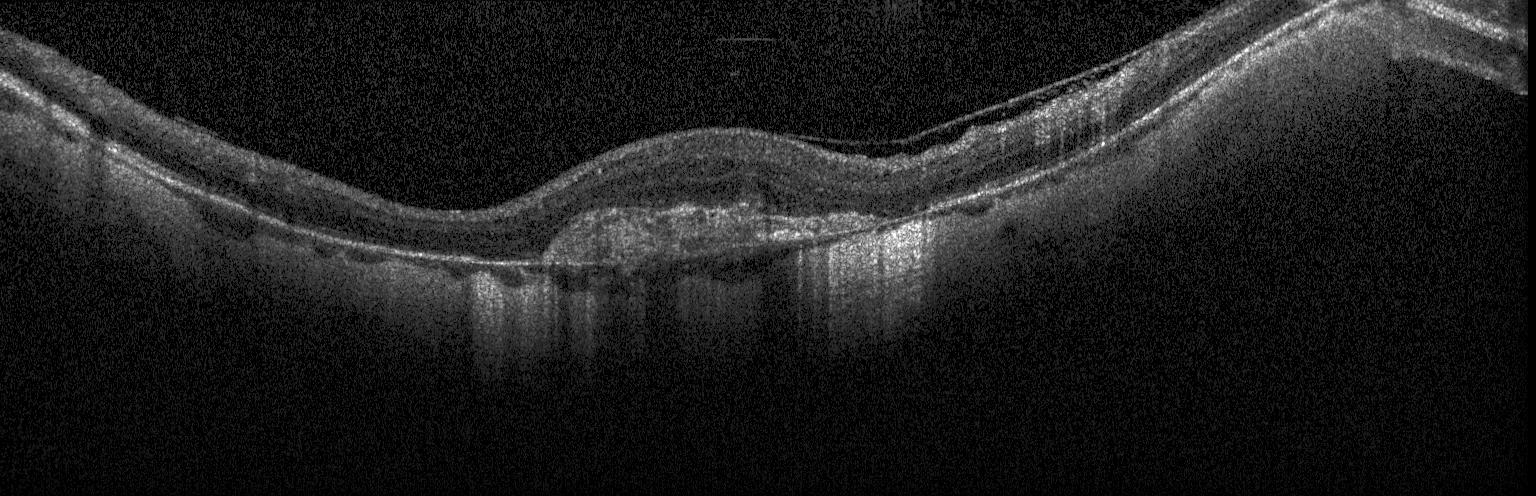
Dx: a choroidal neovascular membrane.